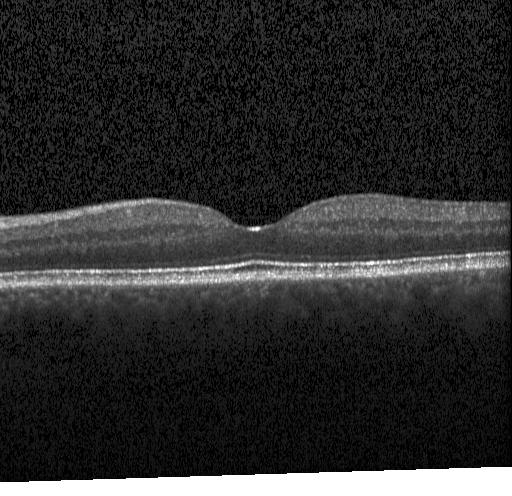 Diagnosis: neither choroidal neovascularization, diabetic macular edema, nor drusen.